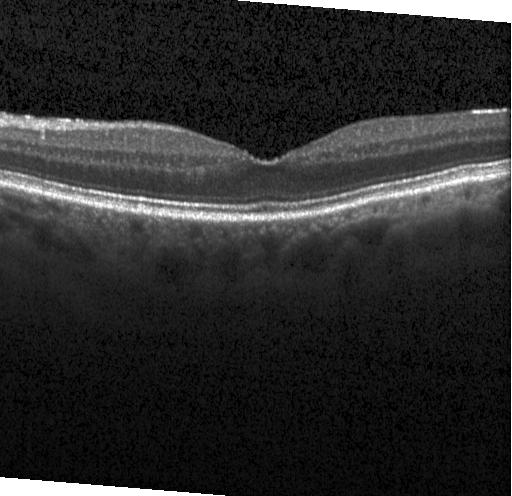
Impression: neither choroidal neovascularization, diabetic macular edema, nor drusen.